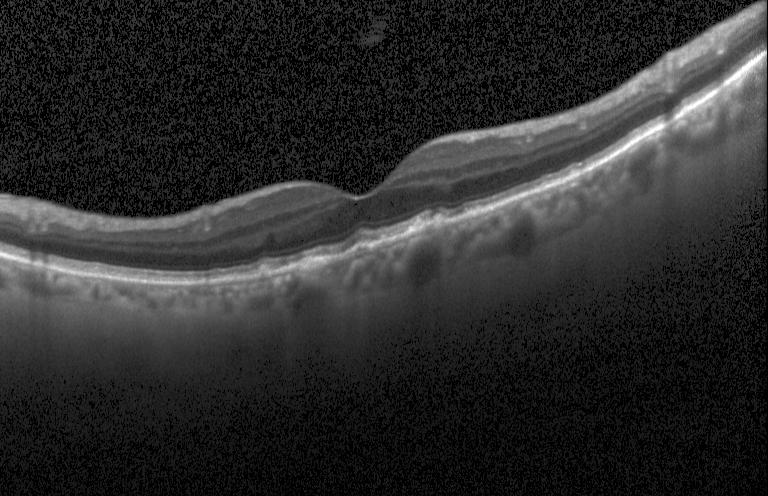

Optical coherence tomography scan; macular scan
Impression: diabetic macular edema (DME).